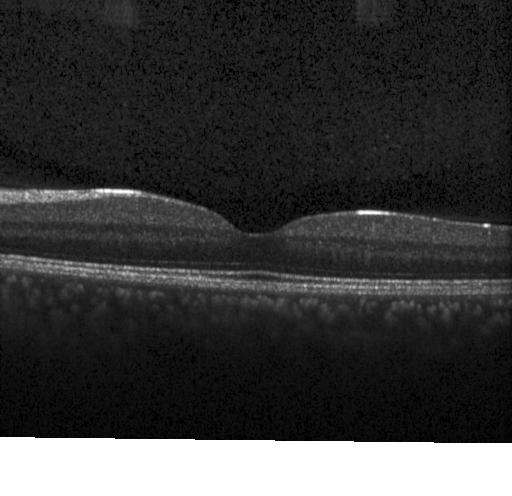

SD-OCT. OCT line scan. Instrument: Heidelberg Spectralis. Horizontal scan through the fovea.
Impression: no CNV, no DME, and no drusen.